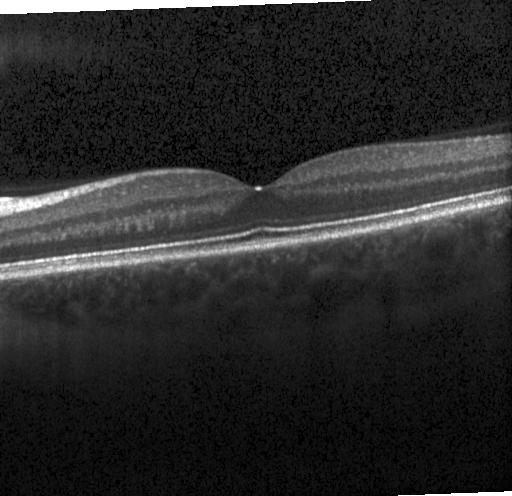

Retinal OCT B-scan; SD-OCT.
OCT finding: neither CNV, DME, nor drusen.